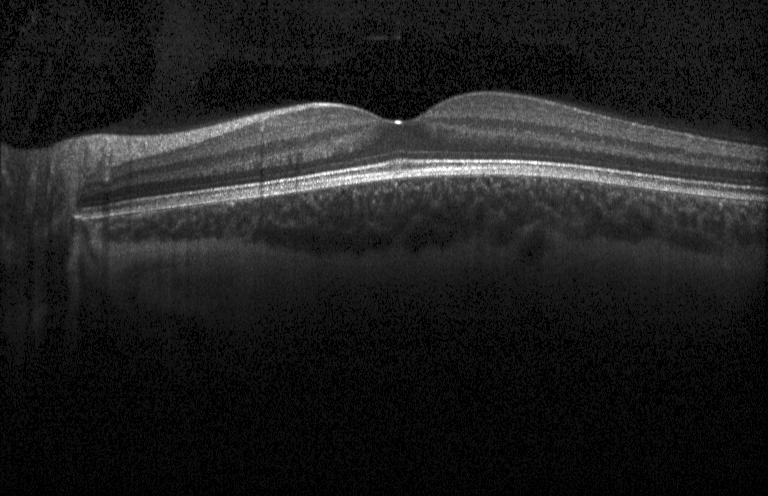

Macular OCT: no choroidal neovascularization, diabetic macular edema, or drusen.